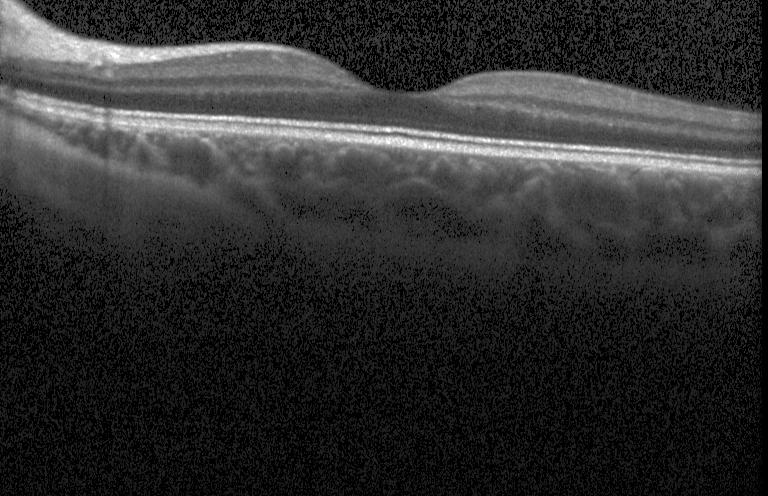

Retinal OCT cross-section; SD-OCT
Impression: neither choroidal neovascularization, diabetic macular edema, nor drusen.